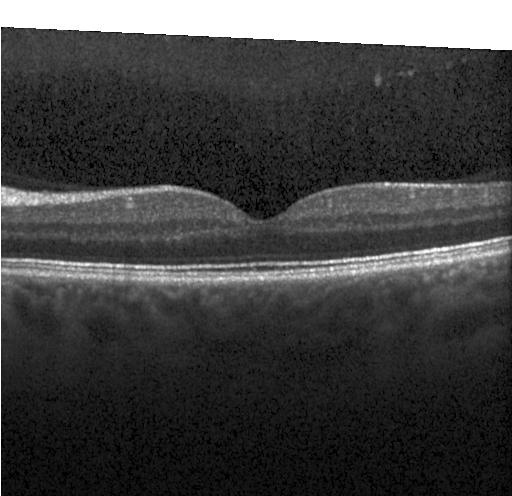 OCT line scan · spectral-domain OCT · instrument: Heidelberg Spectralis · through the macula — Diagnosis: no choroidal neovascularization, no diabetic macular edema, and no drusen.